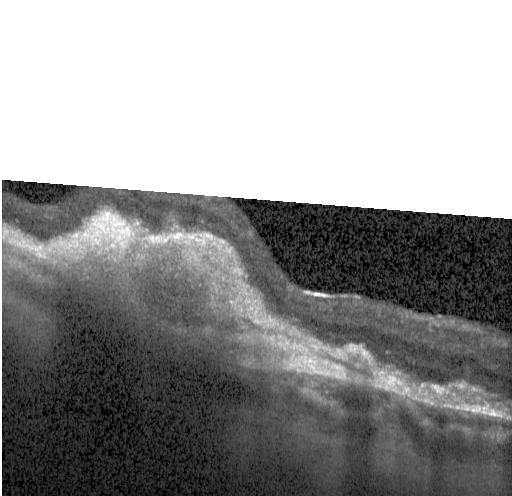 Spectral-domain OCT B-scan: CNV.